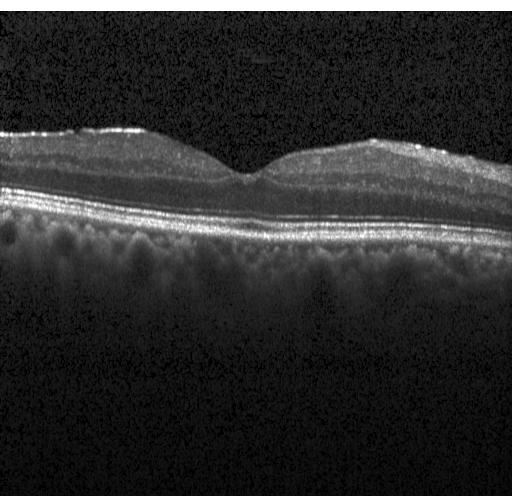 Acquired on a Heidelberg Spectralis, macular scan, optical coherence tomography scan
Impression: no evidence of CNV, DME, or drusen.